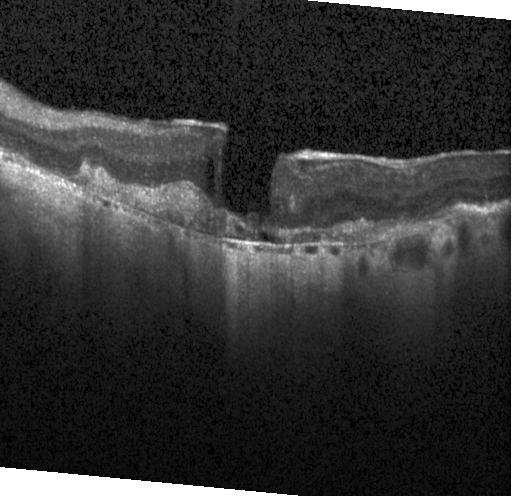 Optical coherence tomography B-scan; spectral-domain OCT. Finding: choroidal neovascularization (CNV).